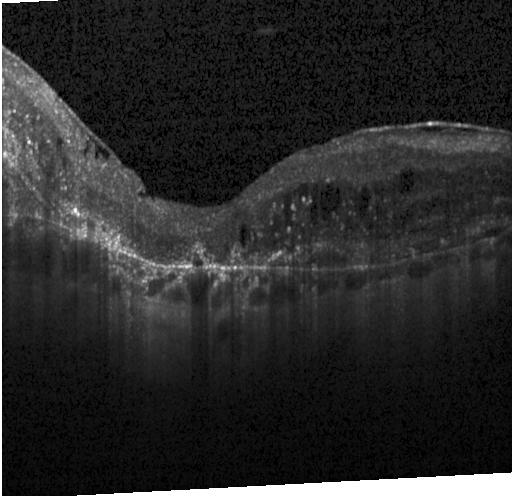
Diagnosis: a choroidal neovascular membrane.